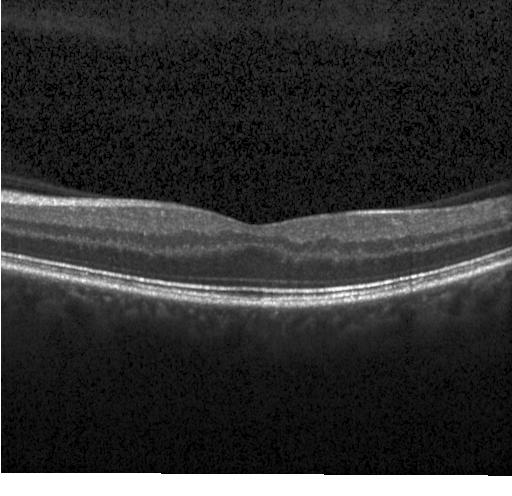 Macular OCT: neither choroidal neovascularization, diabetic macular edema, nor drusen.